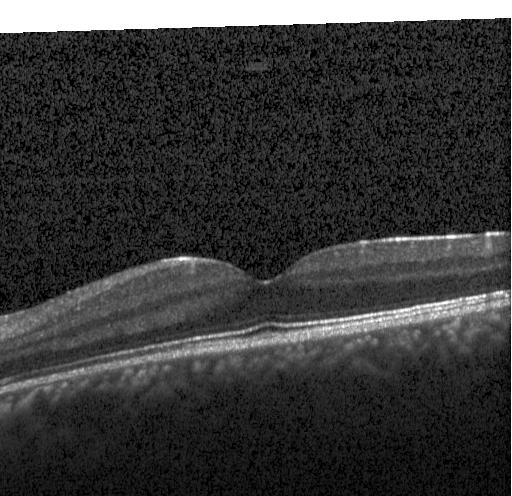

OCT B-scan. OCT finding: no CNV, no DME, and no drusen.